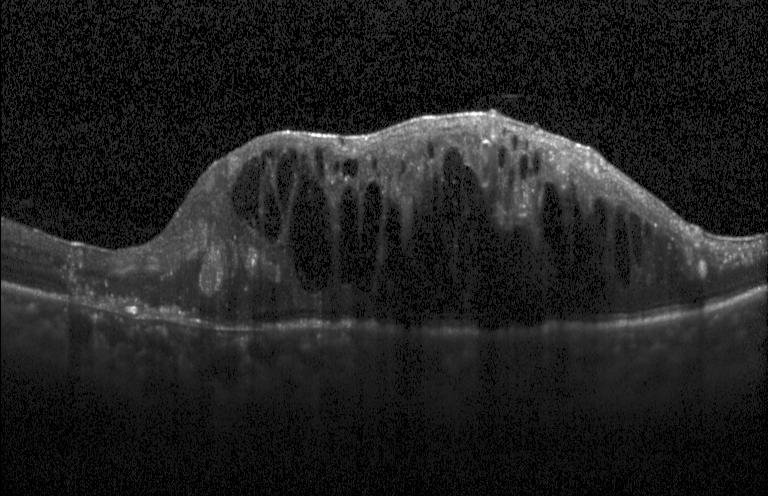
Macular scan · optical coherence tomography B-scan · SD-OCT · instrument: Heidelberg Spectralis
Finding: diabetic macular edema.